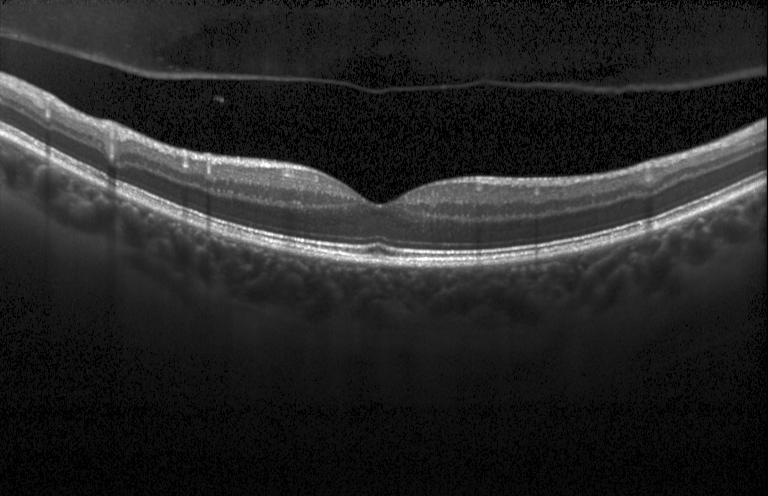

OCT B-scan
Impression: neither choroidal neovascularization, diabetic macular edema, nor drusen.